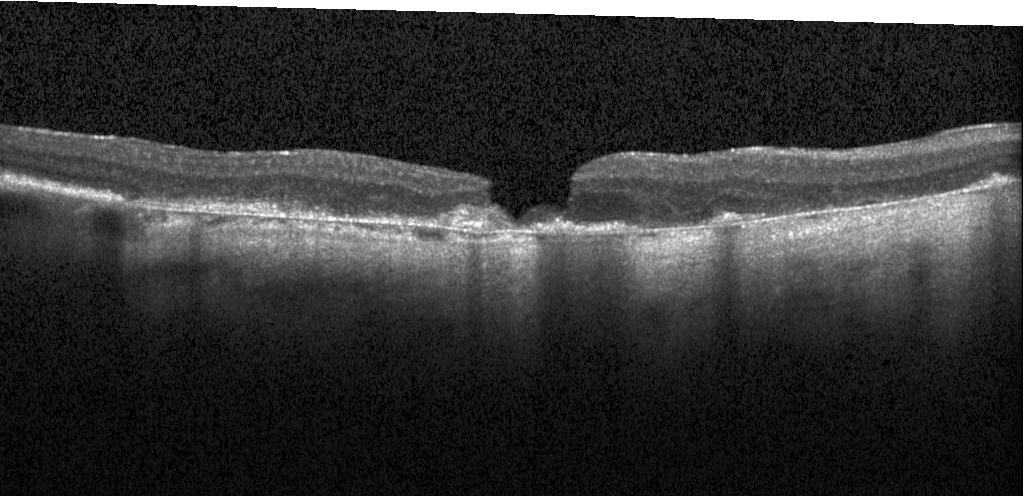 Retinal OCT B-scan · through the macula · acquired on a Heidelberg Spectralis · spectral-domain OCT. Diagnosis: CNV.